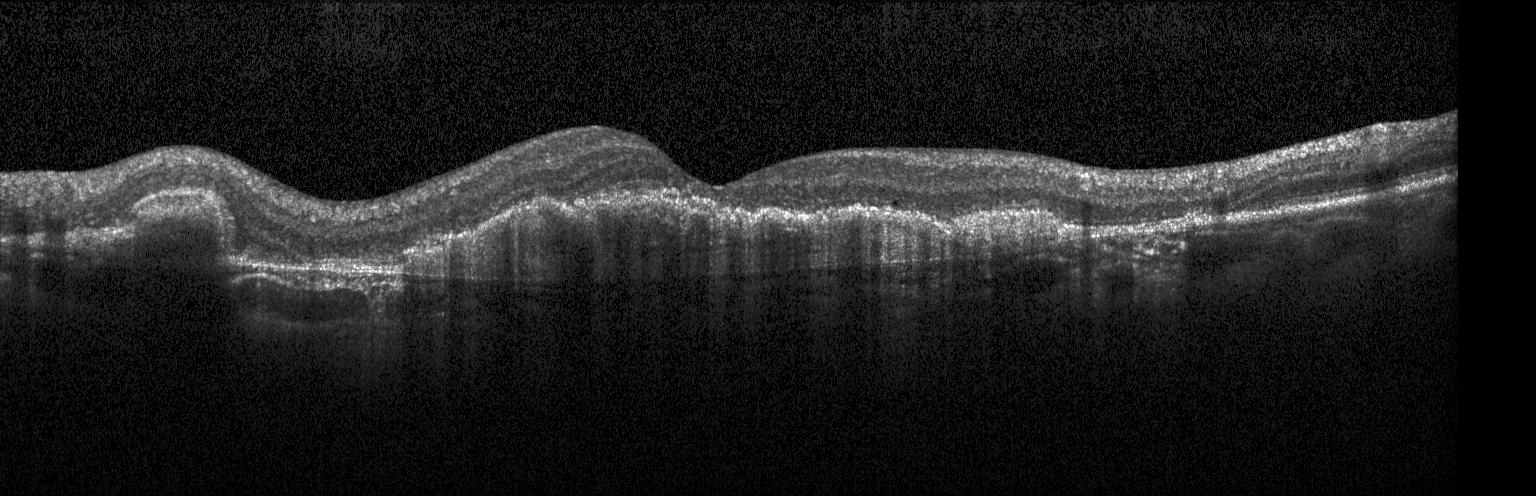

Fovea-centered. OCT B-scan.
Finding: choroidal neovascularization (CNV).